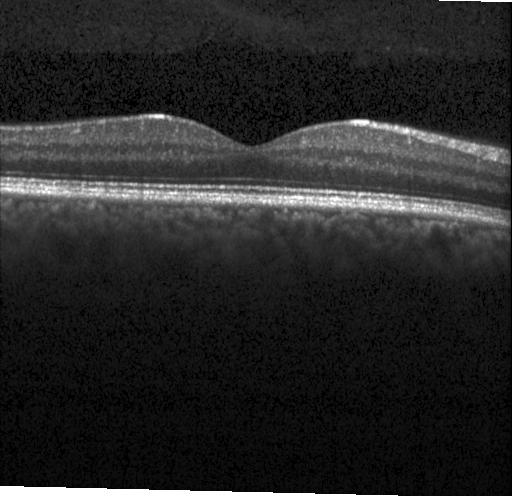
Fovea-centered. SD-OCT. Retinal OCT B-scan. Heidelberg Spectralis. Macular OCT: no evidence of choroidal neovascularization, diabetic macular edema, or drusen.